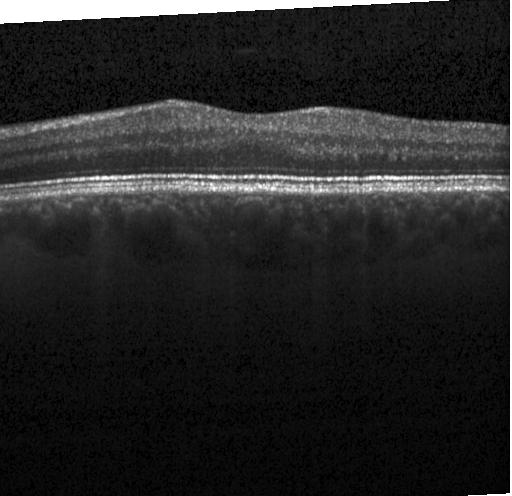
Retinal OCT cross-section showing neither choroidal neovascularization, diabetic macular edema, nor drusen.